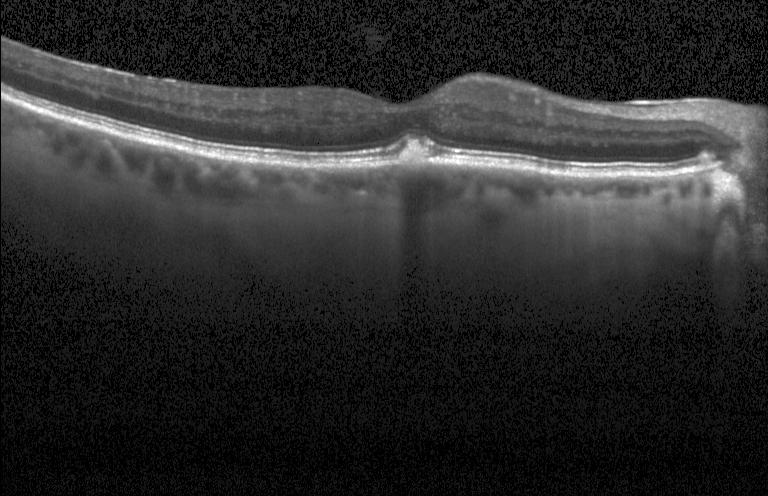 Sub-RPE drusenoid deposits.